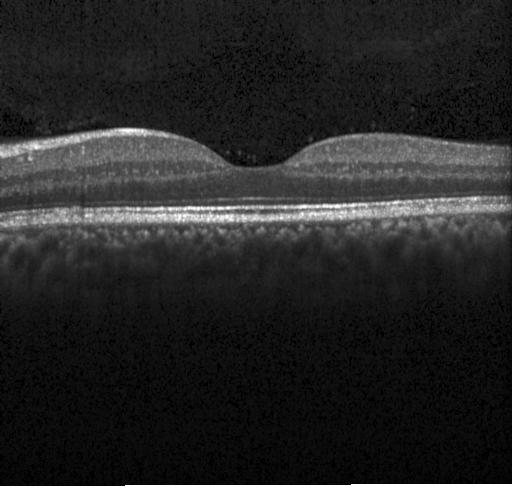

Spectral-domain optical coherence tomography, instrument: Heidelberg Spectralis, retinal OCT cross-section. Finding: no evidence of choroidal neovascularization, diabetic macular edema, or drusen.